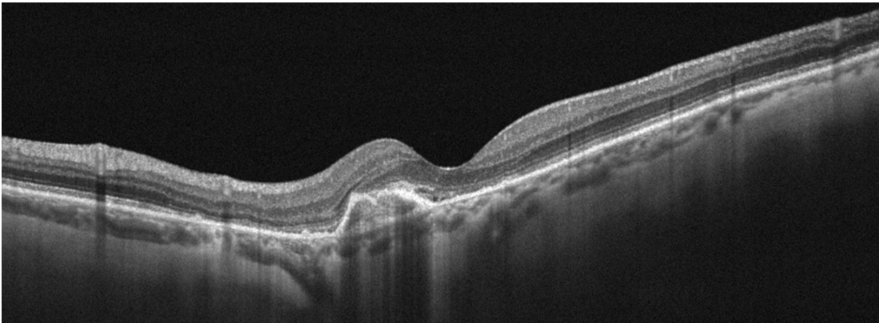
Retinal OCT cross-section. Impression: AMD.